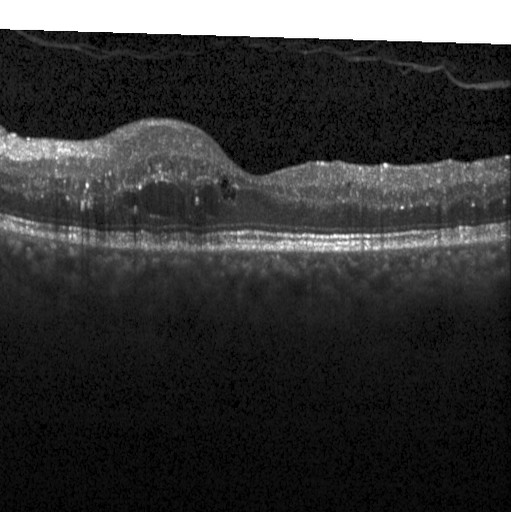 OCT B-scan, instrument: Heidelberg Spectralis, fovea-centered
Finding: diabetic macular edema (DME).